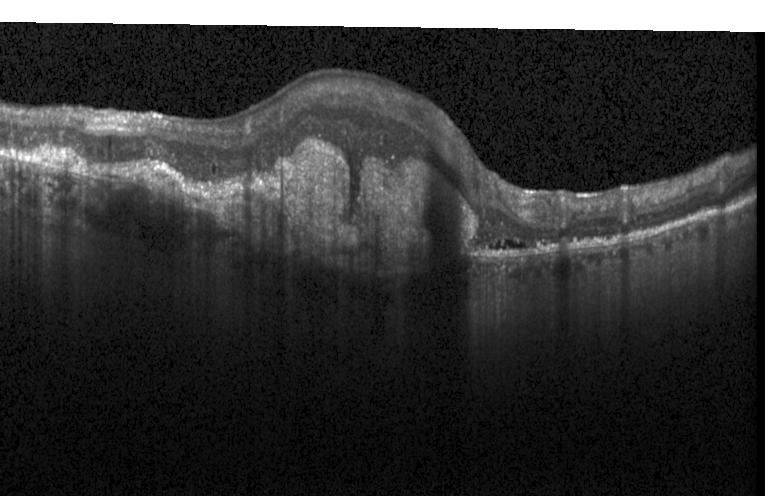 OCT line scan.
Finding: a choroidal neovascular membrane.